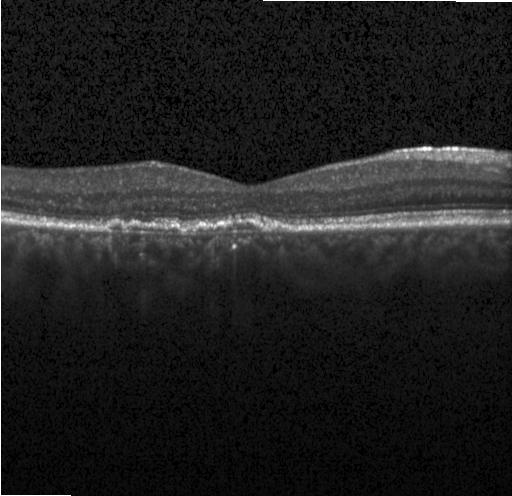

Choroidal neovascularization.